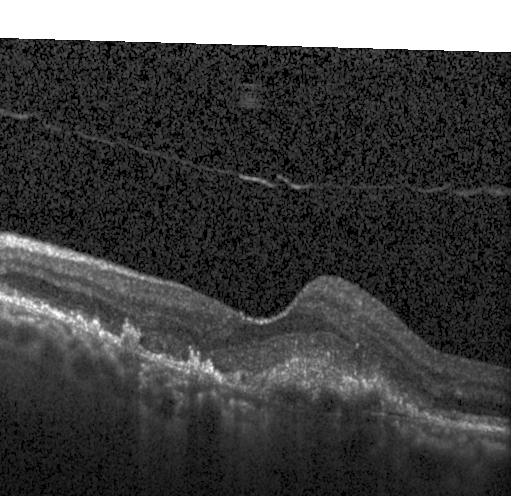

Retinal OCT cross-section — Macular OCT: a choroidal neovascular membrane.